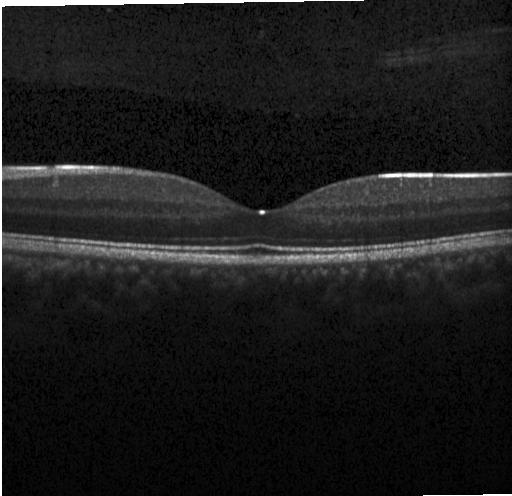 Spectral-domain OCT; optical coherence tomography B-scan; through the macula; instrument: Heidelberg Spectralis.
Impression: no evidence of choroidal neovascularization, diabetic macular edema, or drusen.